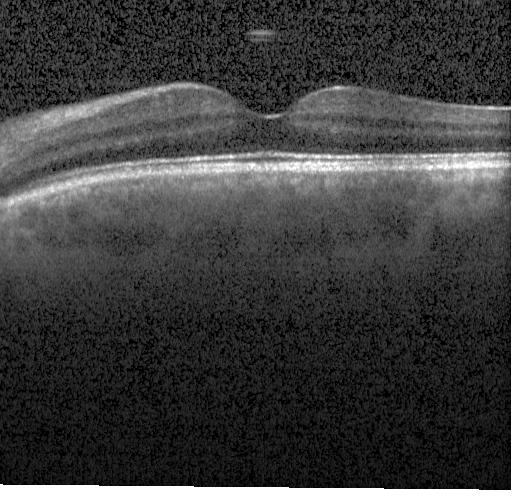

Diagnosis: no CNV, DME, or drusen.